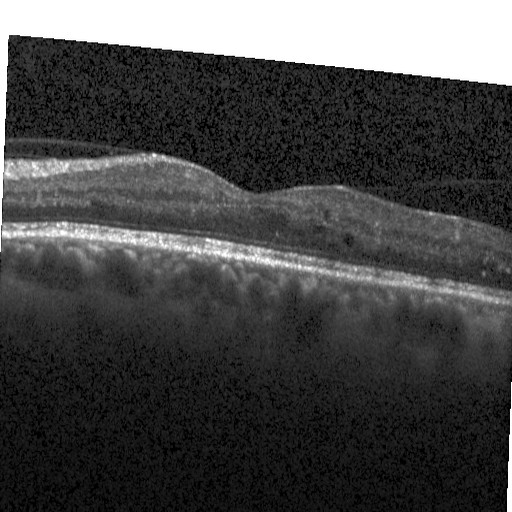 This B-scan demonstrates diabetic macular edema.